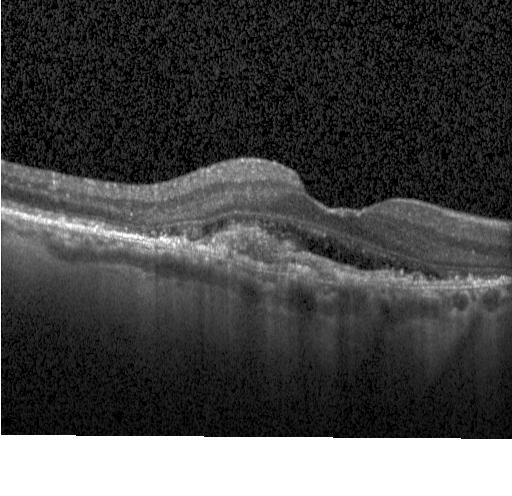
A choroidal neovascular membrane.